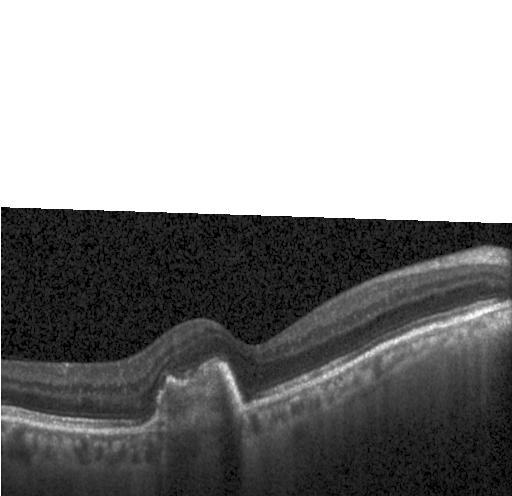

Retinal OCT cross-section · acquired on a Heidelberg Spectralis. Impression: a choroidal neovascular membrane.